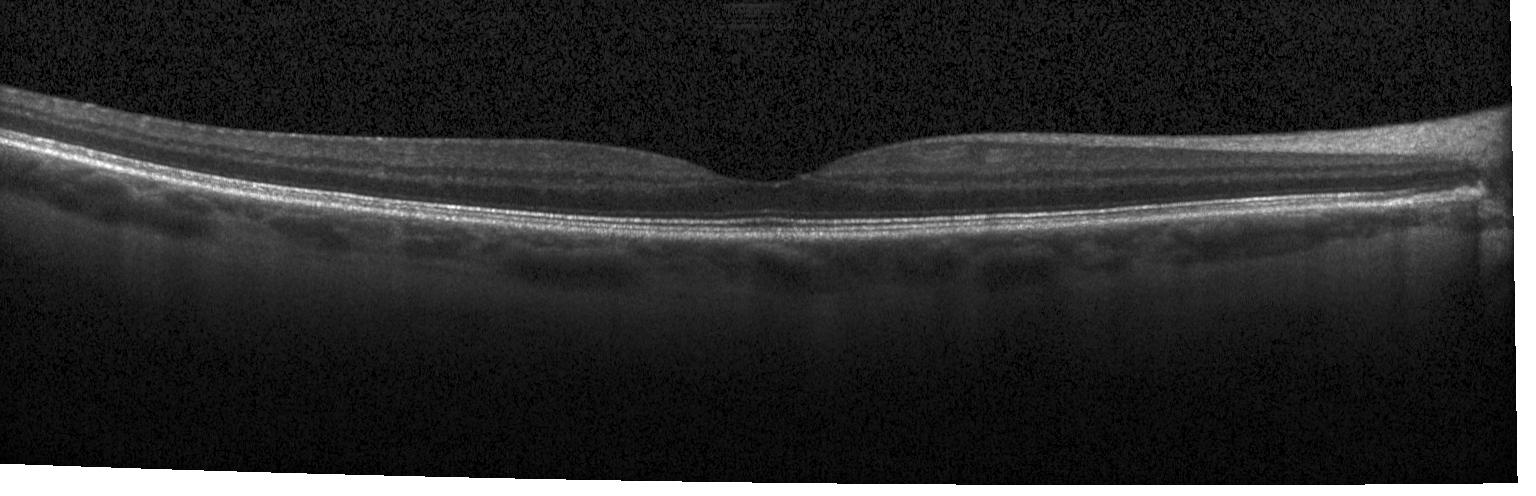 Retinal OCT cross-section. Heidelberg Spectralis OCT system.
Diagnosis: no choroidal neovascularization, diabetic macular edema, or drusen.